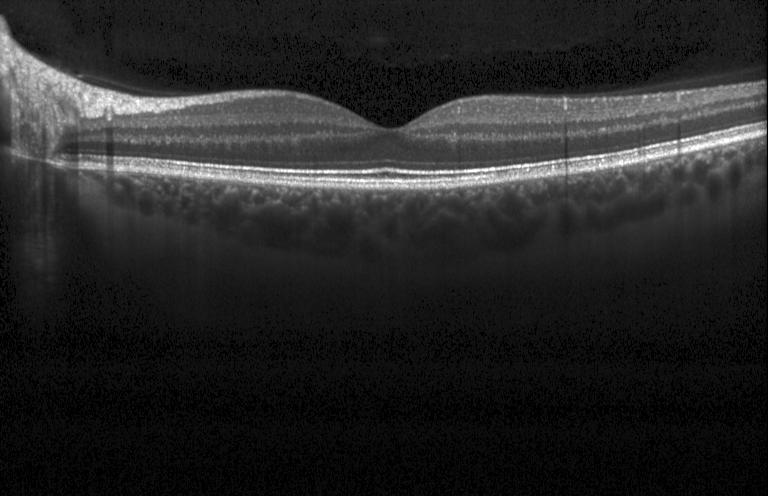 Spectral-domain OCT. Optical coherence tomography scan. Assessment: neither choroidal neovascularization, diabetic macular edema, nor drusen.